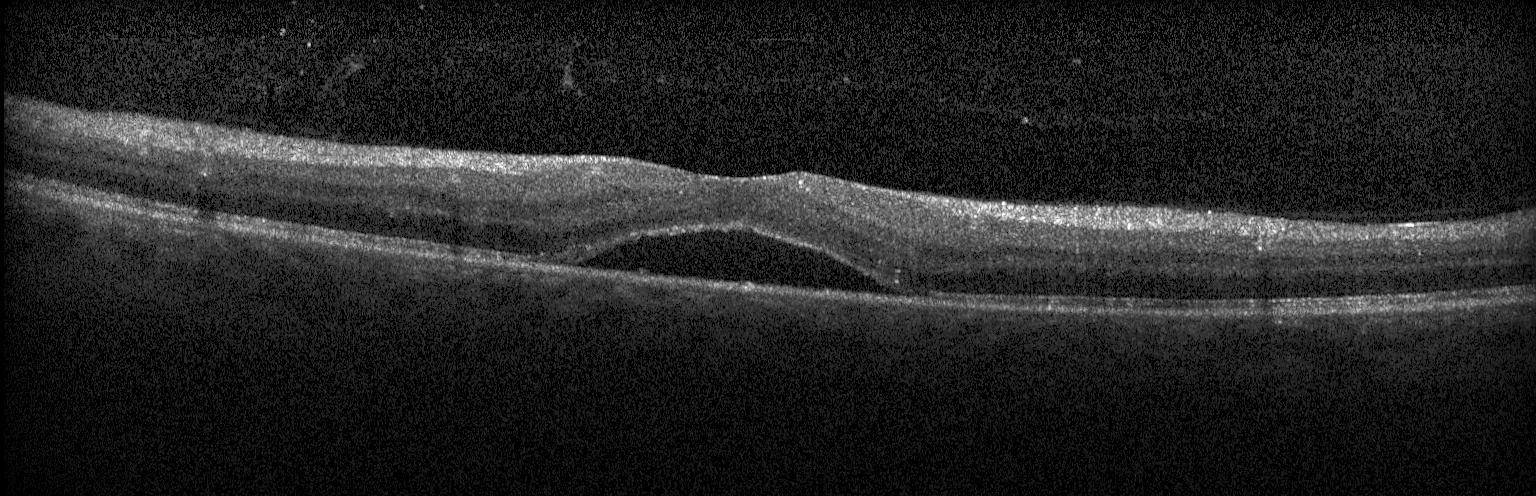
Spectral-domain OCT B-scan: CNV.